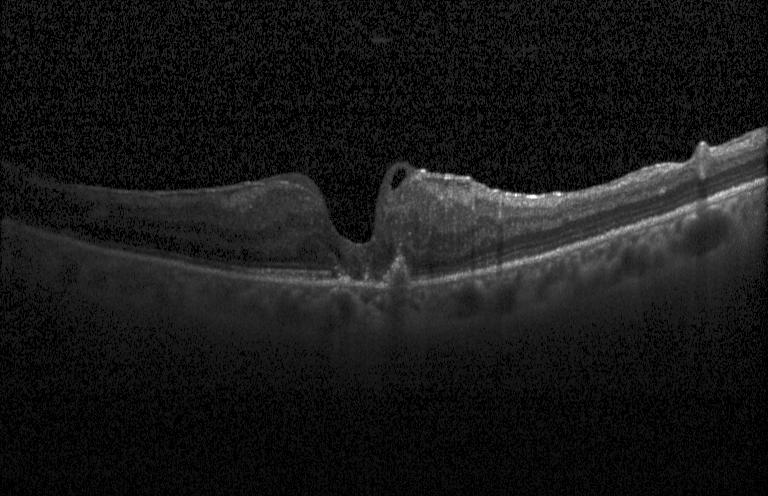 Dx: diabetic macular edema (DME).